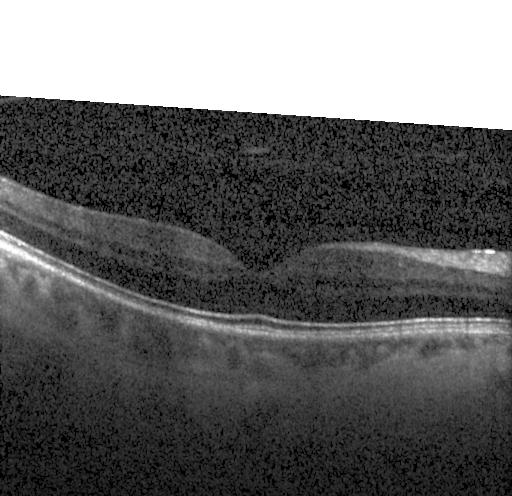 Heidelberg Spectralis OCT system, macular scan, optical coherence tomography B-scan, spectral-domain OCT. Neither CNV, DME, nor drusen.